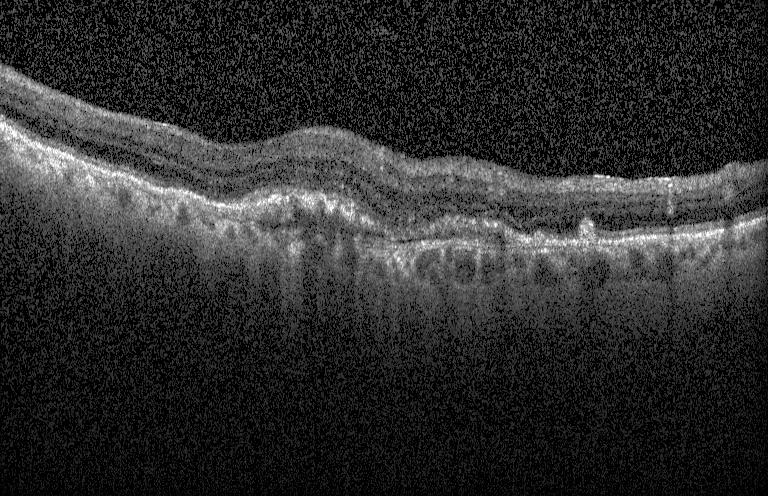

Optical coherence tomography scan
Choroidal neovascularization.